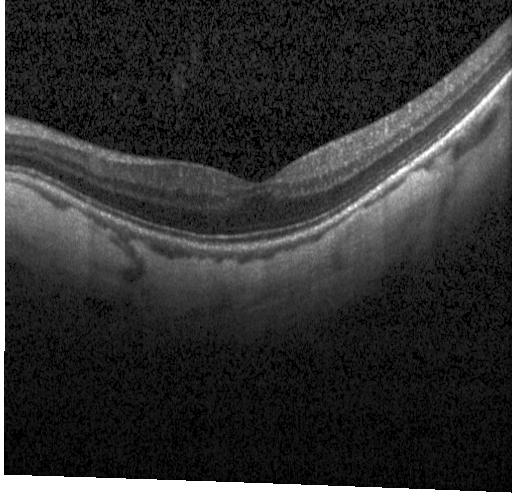

Fovea-centered, Heidelberg Spectralis, optical coherence tomography B-scan, SD-OCT.
Dx: no choroidal neovascularization, no diabetic macular edema, and no drusen.